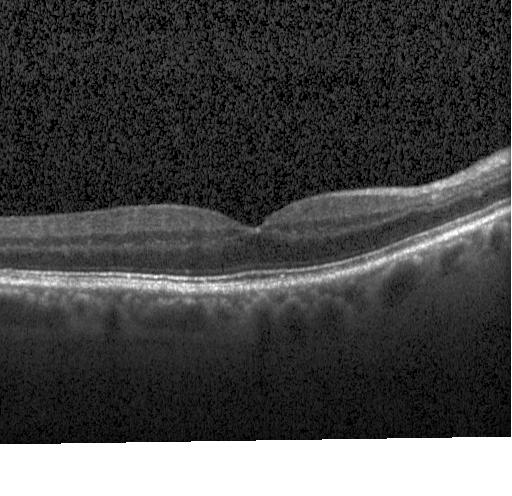

Optical coherence tomography scan. SD-OCT
Impression: no choroidal neovascularization, diabetic macular edema, or drusen.